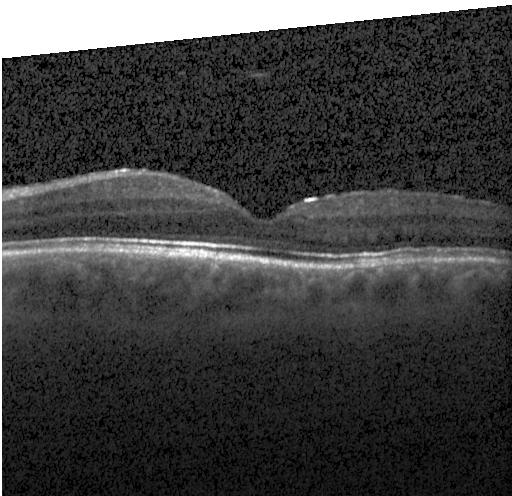
Retinal OCT cross-section. Spectral-domain OCT. Heidelberg Spectralis
Finding: no evidence of choroidal neovascularization, diabetic macular edema, or drusen.